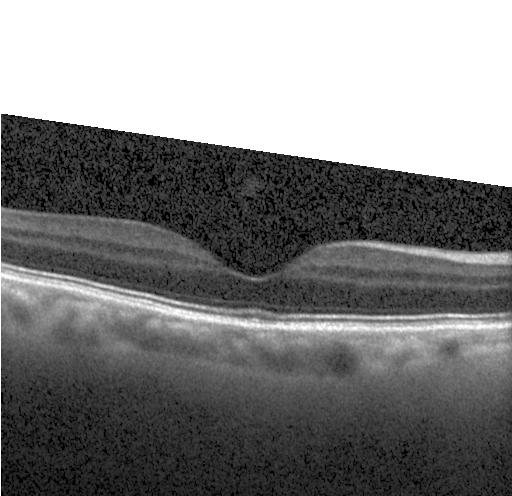
Macular OCT: no CNV, no DME, and no drusen.